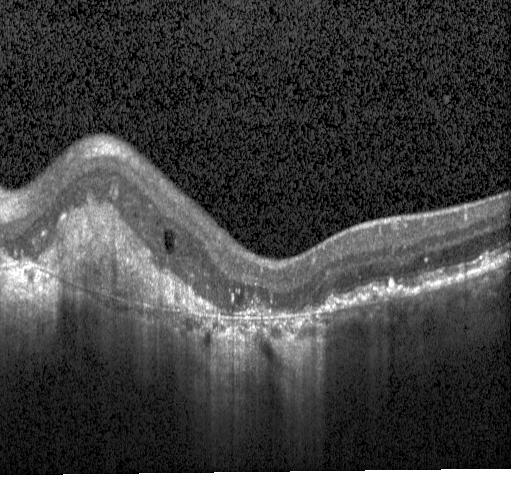
Diagnosis: a choroidal neovascular membrane.